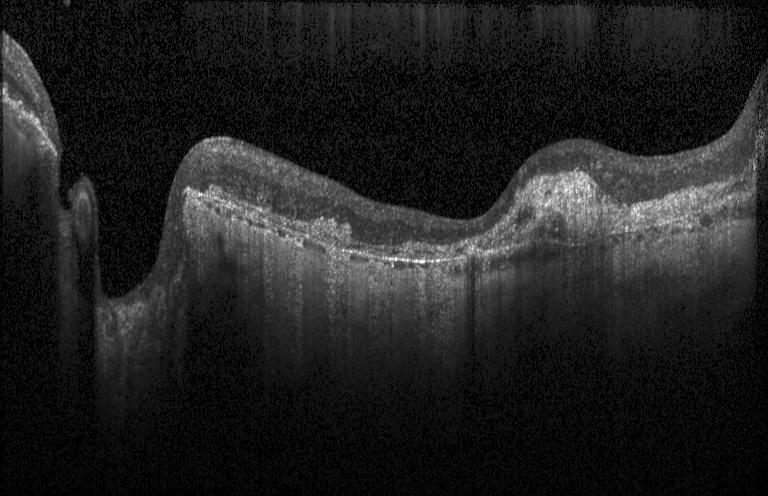
OCT B-scan, horizontal scan through the fovea
Impression: choroidal neovascularization (CNV).